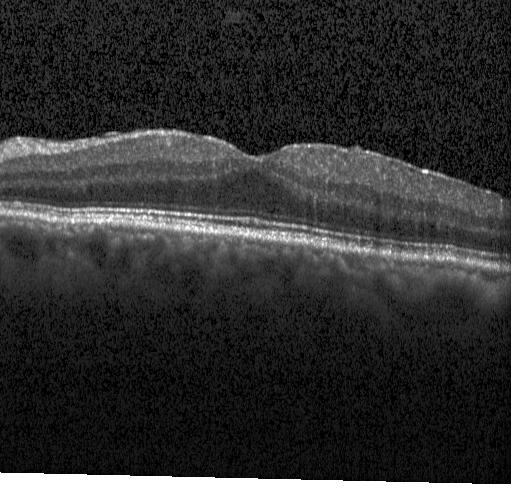

Dx: no choroidal neovascularization, diabetic macular edema, or drusen.